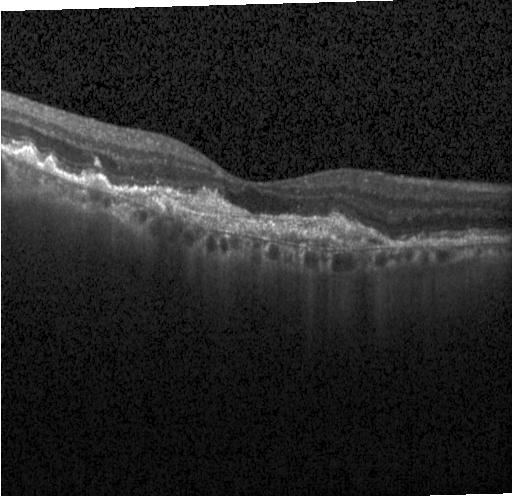 OCT B-scan showing choroidal neovascularization.